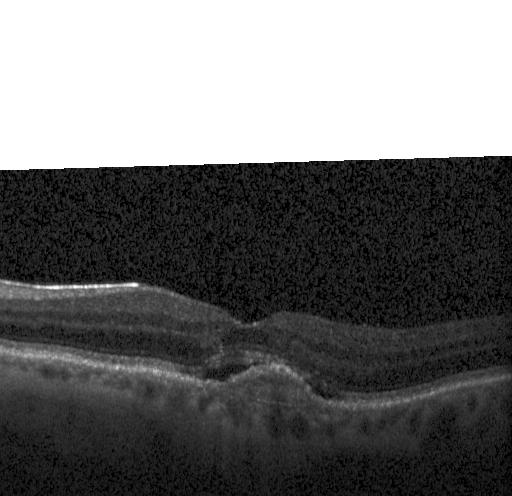
OCT line scan
This B-scan demonstrates a choroidal neovascular membrane.